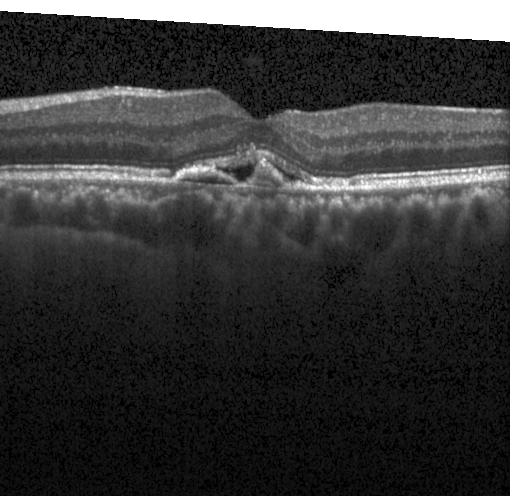

SD-OCT, optical coherence tomography B-scan.
Macular OCT: CNV.